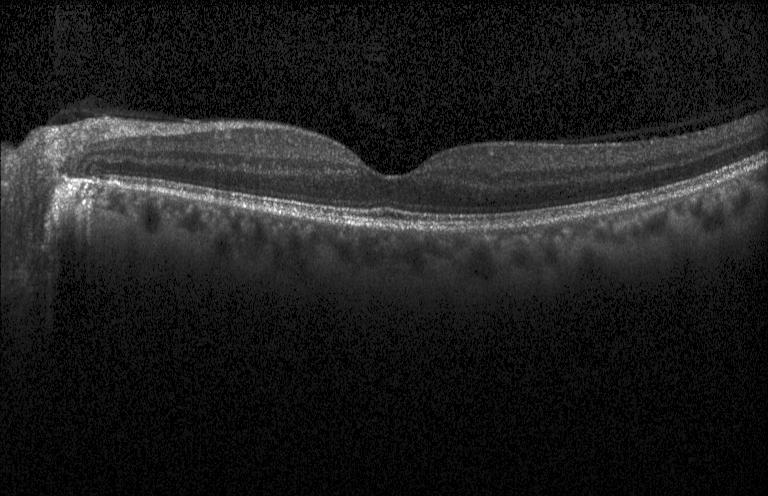

Optical coherence tomography B-scan. Finding: no CNV, no DME, and no drusen.